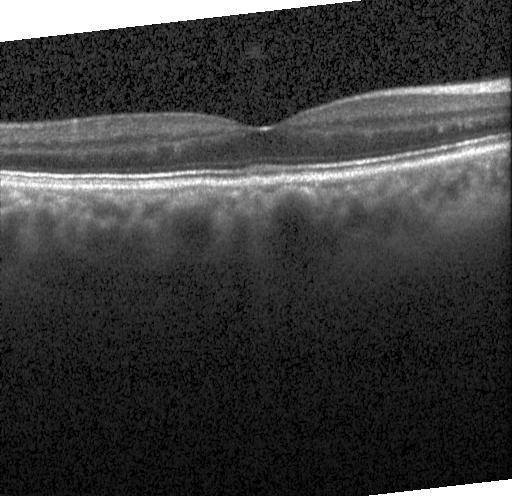

Spectral-domain optical coherence tomography, macular scan, acquired on a Heidelberg Spectralis, retinal OCT cross-section — Macular OCT: neither choroidal neovascularization, diabetic macular edema, nor drusen.